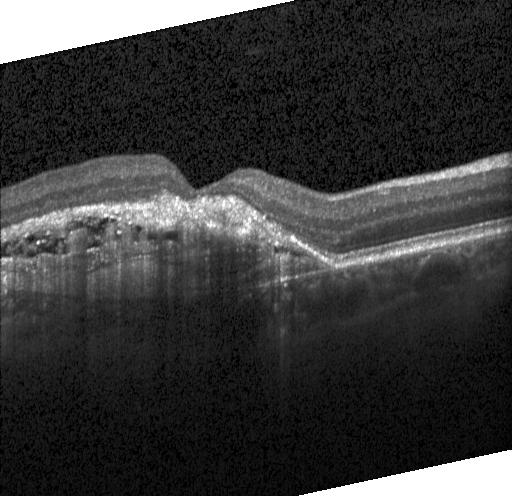 Retinal OCT cross-section · macular scan. Diagnosis: choroidal neovascularization.